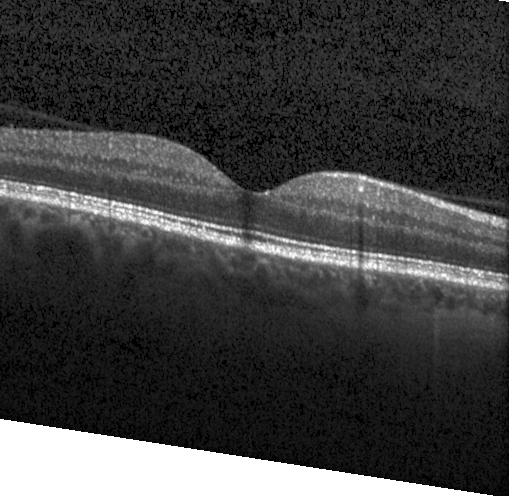 The scan shows neither CNV, DME, nor drusen.